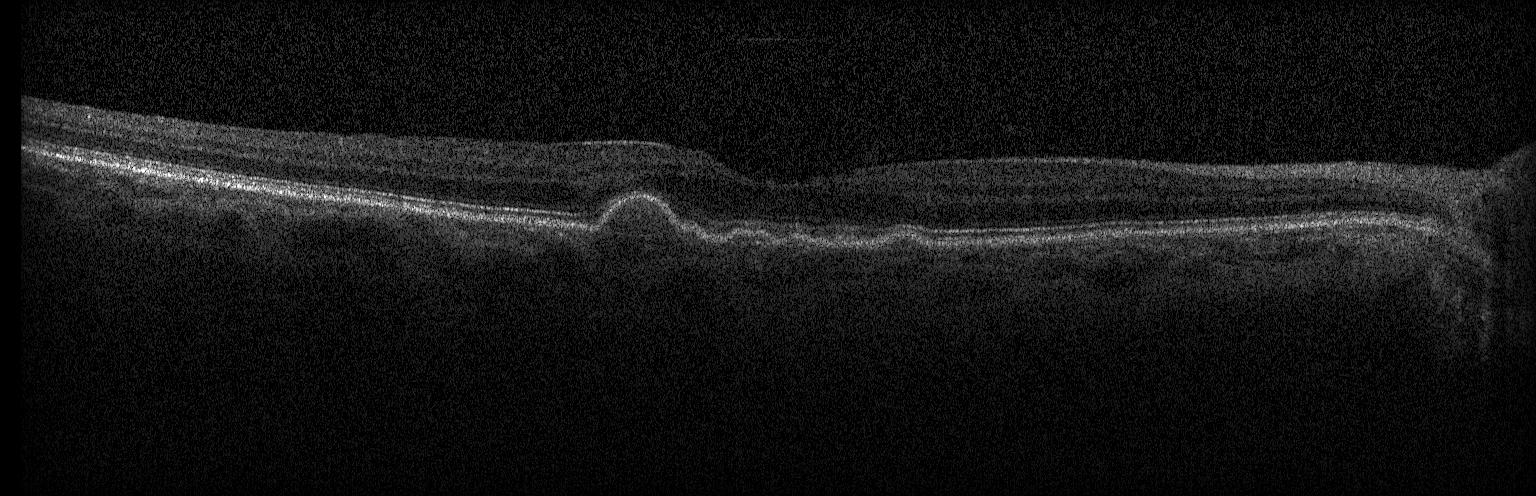

Spectral-domain OCT · fovea-centered · retinal OCT B-scan
Finding: drusen.